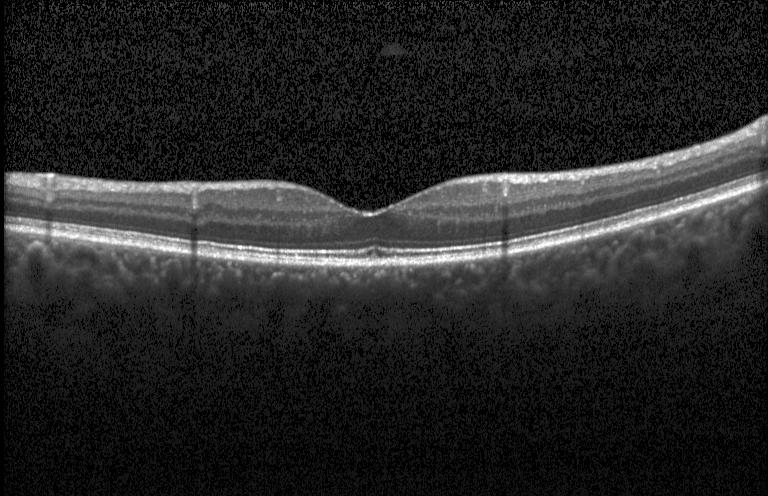
Acquired on a Heidelberg Spectralis · optical coherence tomography B-scan · SD-OCT.
Diagnosis: neither choroidal neovascularization, diabetic macular edema, nor drusen.